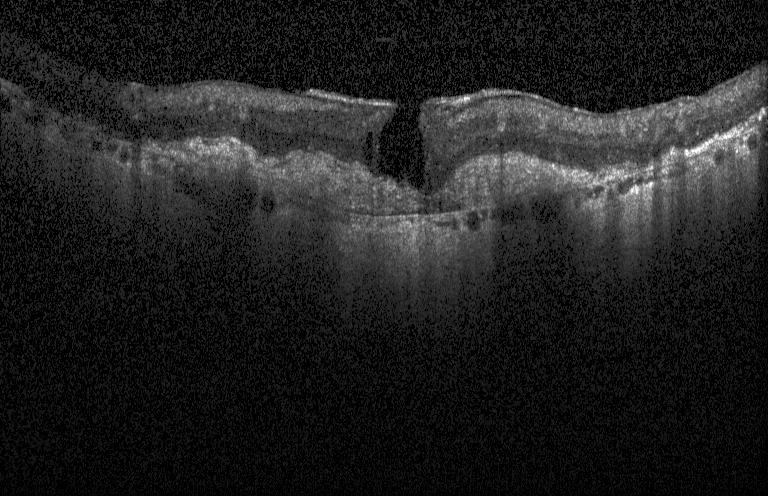
OCT finding: a choroidal neovascular membrane.